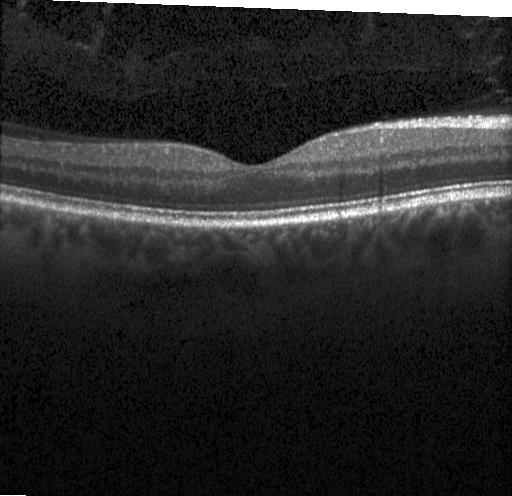 Horizontal scan through the fovea · SD-OCT · instrument: Heidelberg Spectralis · retinal OCT B-scan. This B-scan demonstrates no choroidal neovascularization, no diabetic macular edema, and no drusen.